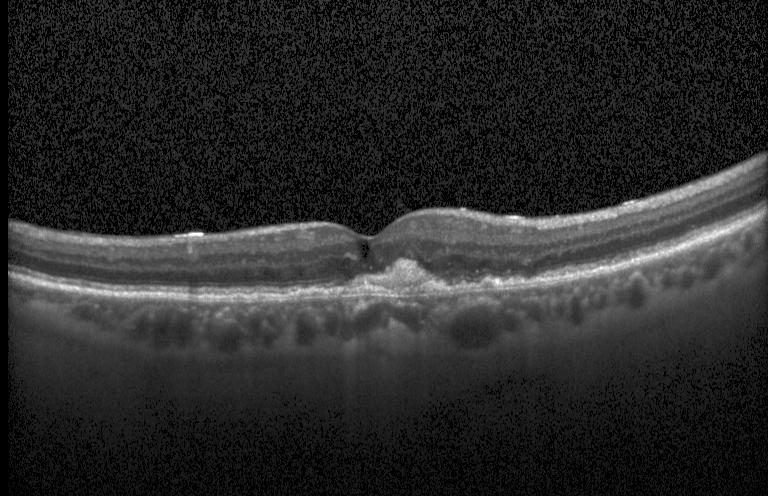 Impression: choroidal neovascularization.